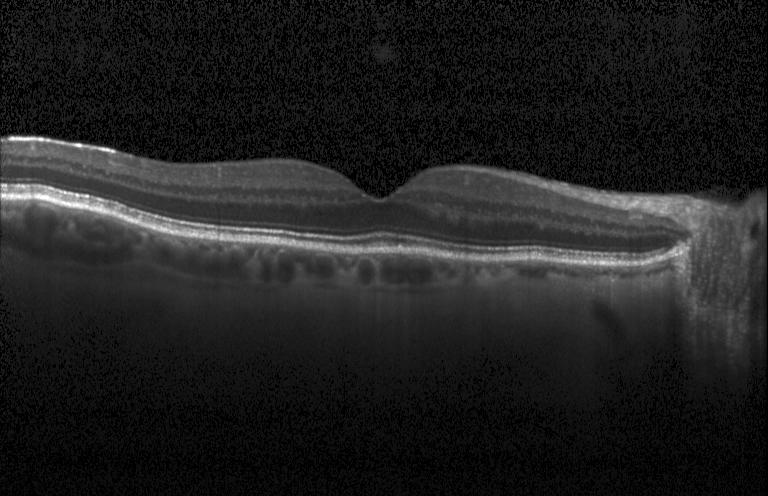 Through the macula · retinal OCT B-scan.
Finding: no choroidal neovascularization, diabetic macular edema, or drusen.